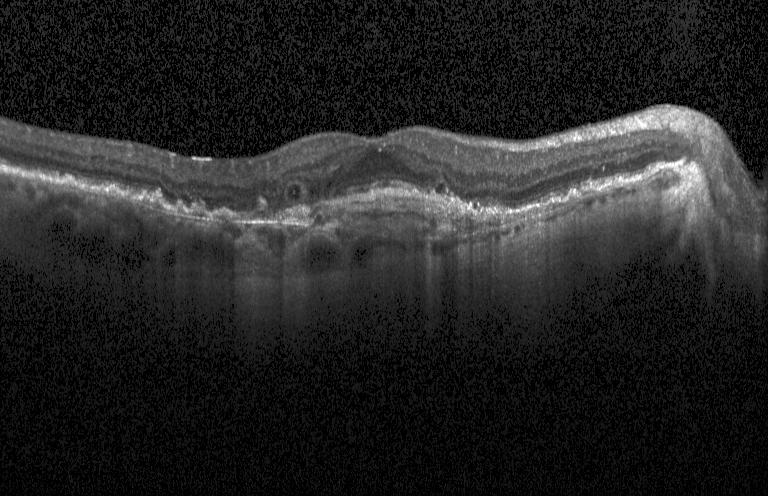 Optical coherence tomography scan · spectral-domain optical coherence tomography · acquired on a Heidelberg Spectralis — Impression: a choroidal neovascular membrane.